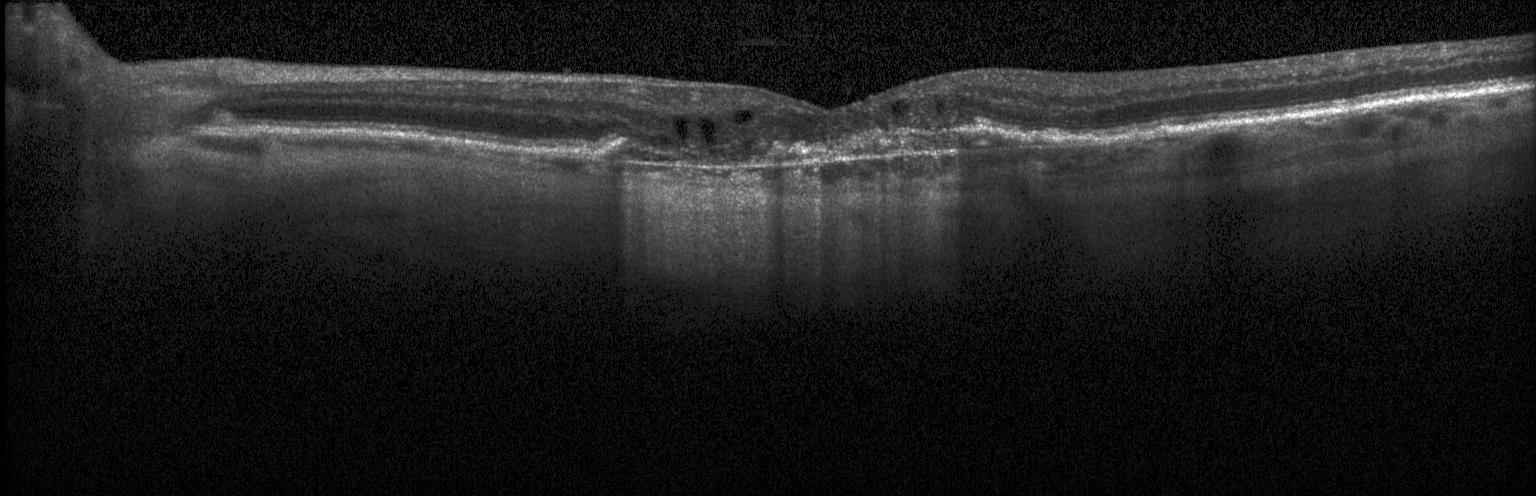

OCT B-scan showing choroidal neovascularization (CNV).